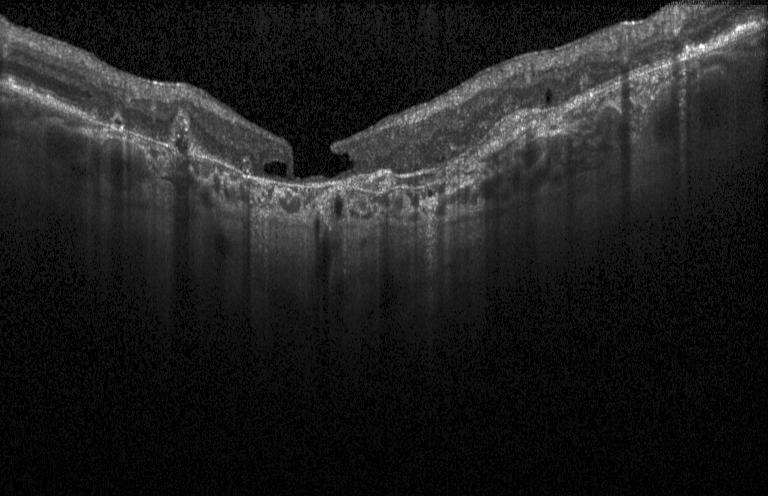
This B-scan demonstrates a choroidal neovascular membrane.